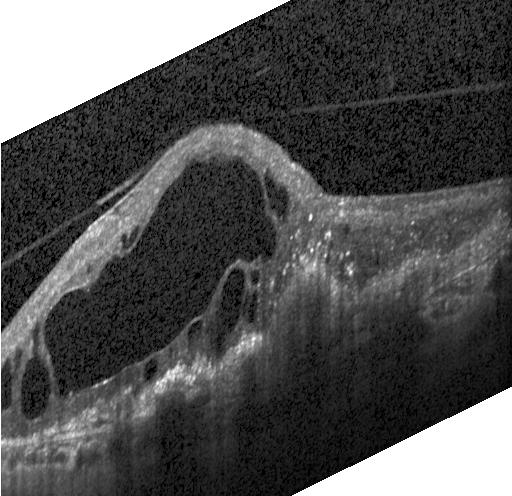
Heidelberg Spectralis OCT system. Spectral-domain optical coherence tomography. Retinal OCT cross-section. Fovea-centered — CNV.